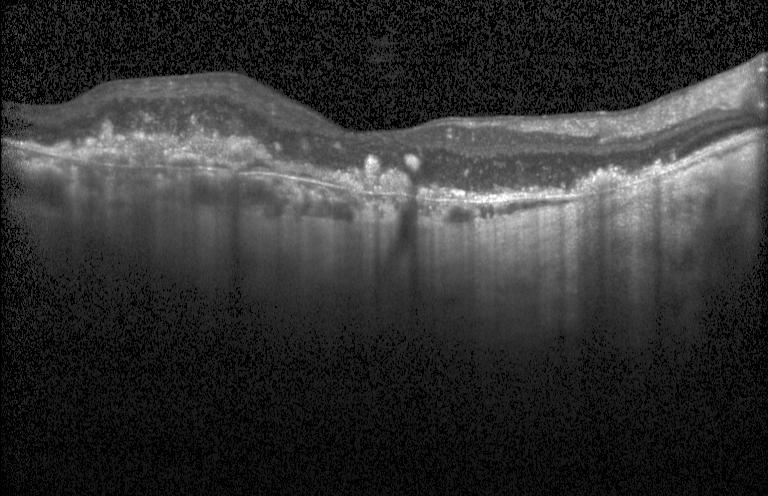 Optical coherence tomography B-scan. Spectral-domain optical coherence tomography
Diagnosis: a choroidal neovascular membrane.